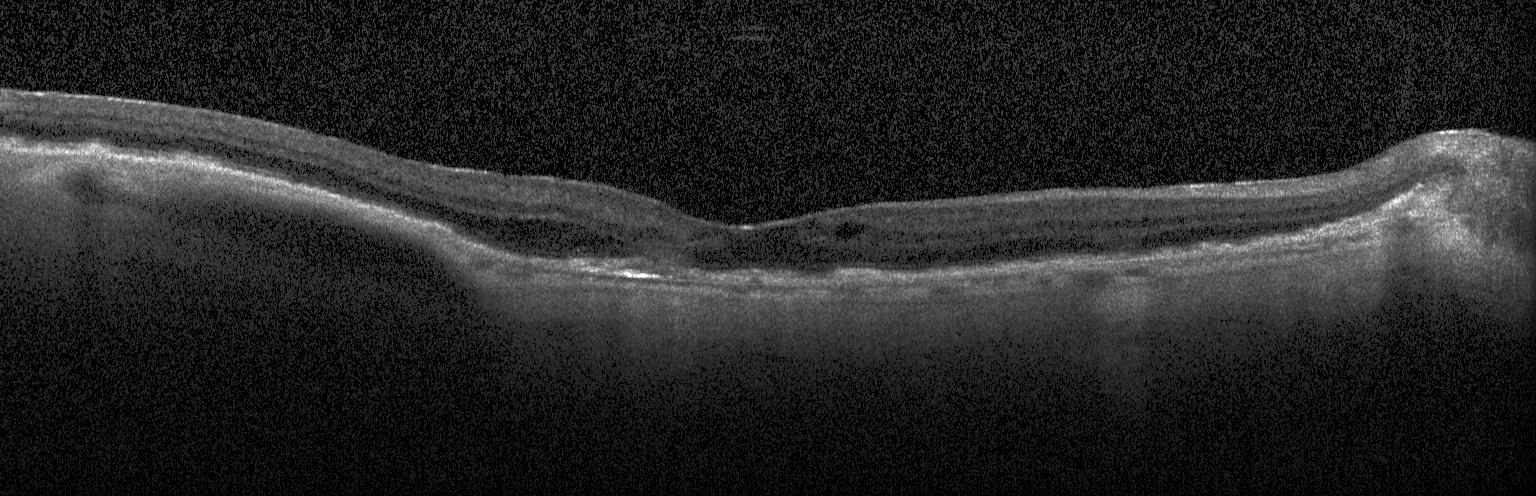
Diagnosis: CNV.